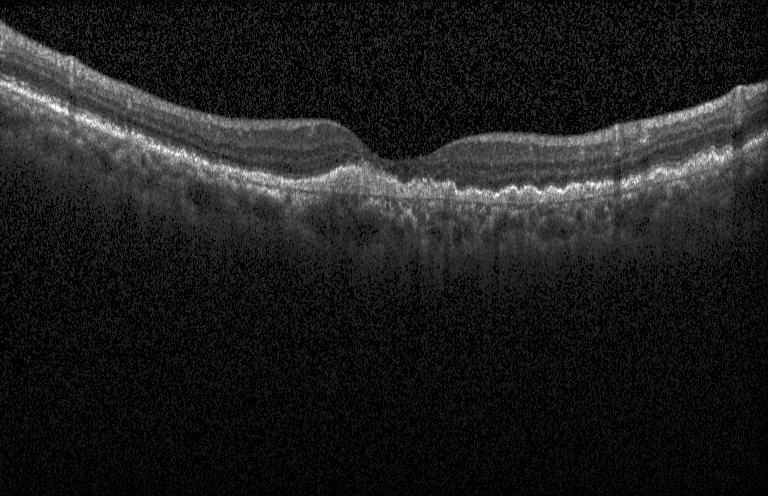

Instrument: Heidelberg Spectralis · OCT line scan · macular scan · spectral-domain optical coherence tomography.
Assessment: CNV.